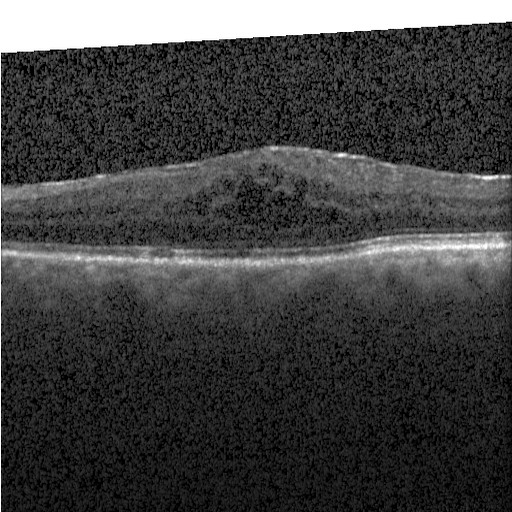
OCT B-scan
Finding: diabetic macular edema (DME).